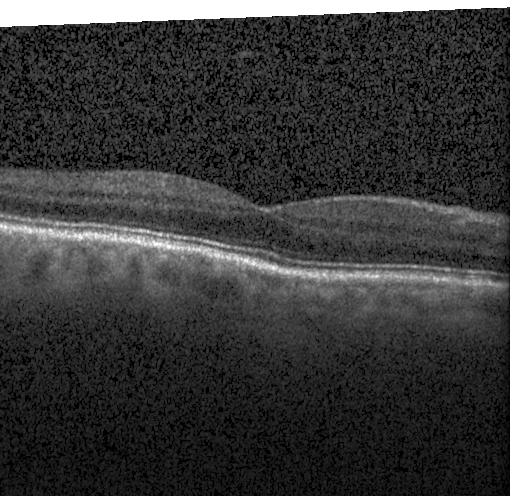 OCT B-scan showing no choroidal neovascularization, no diabetic macular edema, and no drusen.